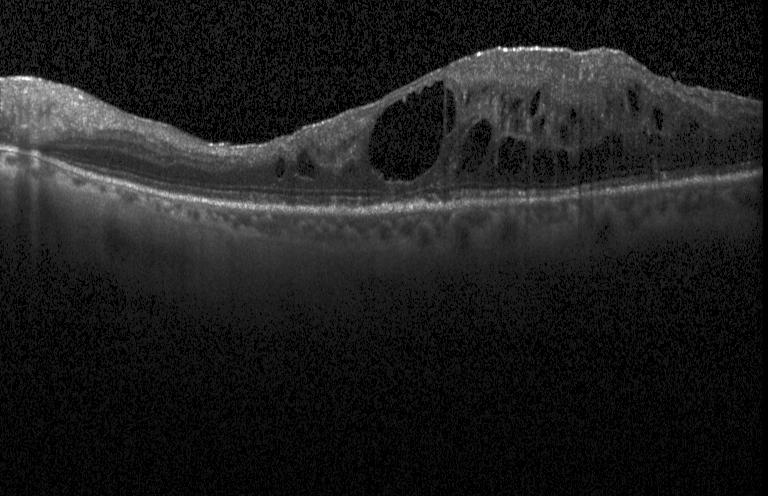
Impression: diabetic macular edema.